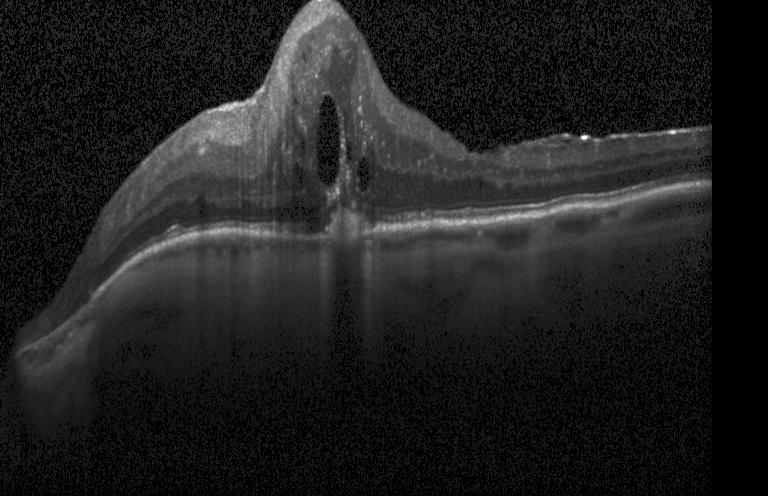 Spectral-domain OCT, optical coherence tomography B-scan — Dx: choroidal neovascularization (CNV).